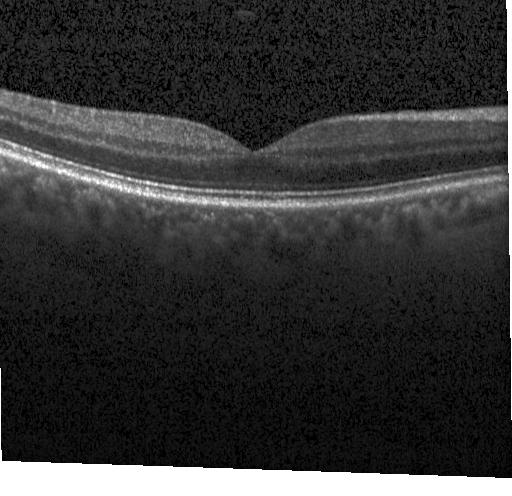
Spectral-domain OCT · OCT line scan · horizontal scan through the fovea. Macular OCT: no evidence of choroidal neovascularization, diabetic macular edema, or drusen.